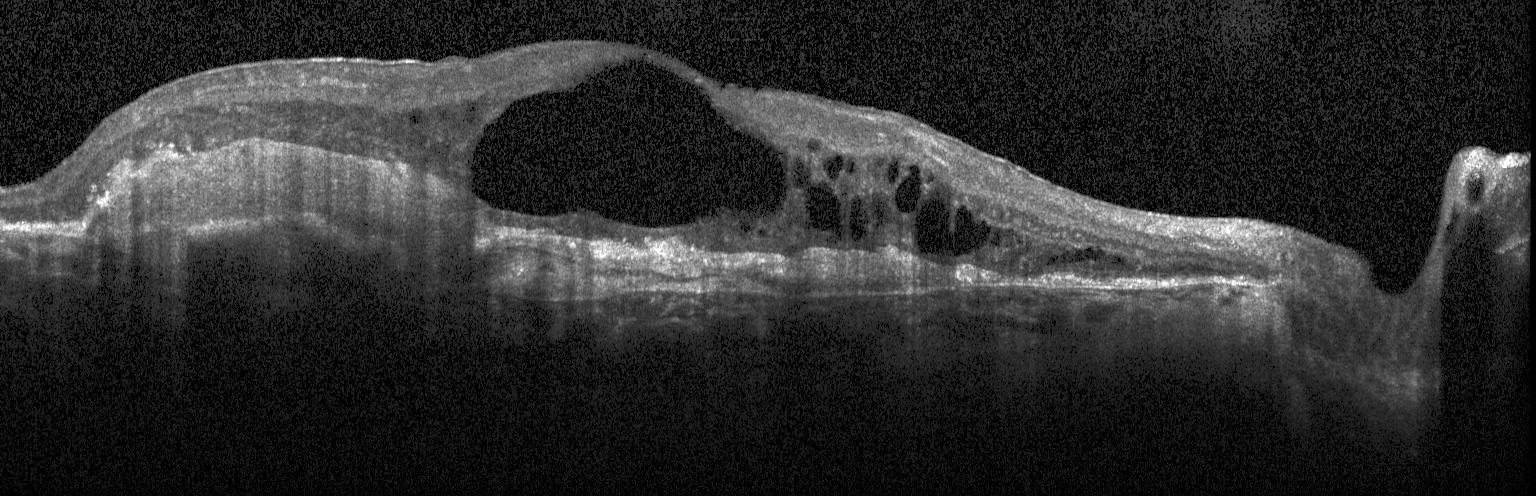
The scan shows a choroidal neovascular membrane.